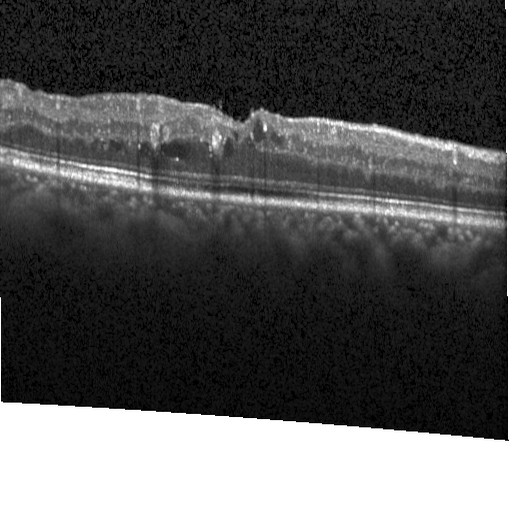
Dx: diabetic macular edema.